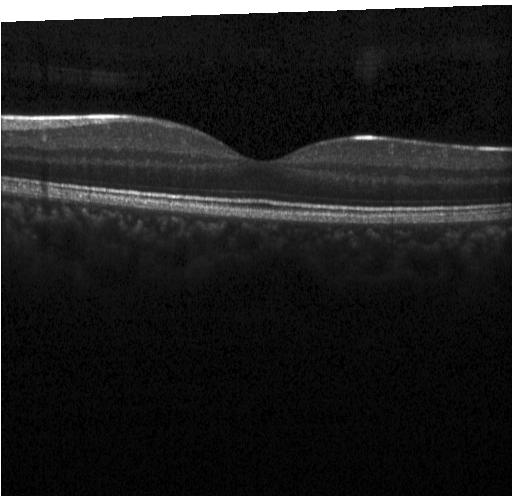
Heidelberg Spectralis · retinal OCT cross-section · macular scan · SD-OCT — Assessment: no choroidal neovascularization, diabetic macular edema, or drusen.